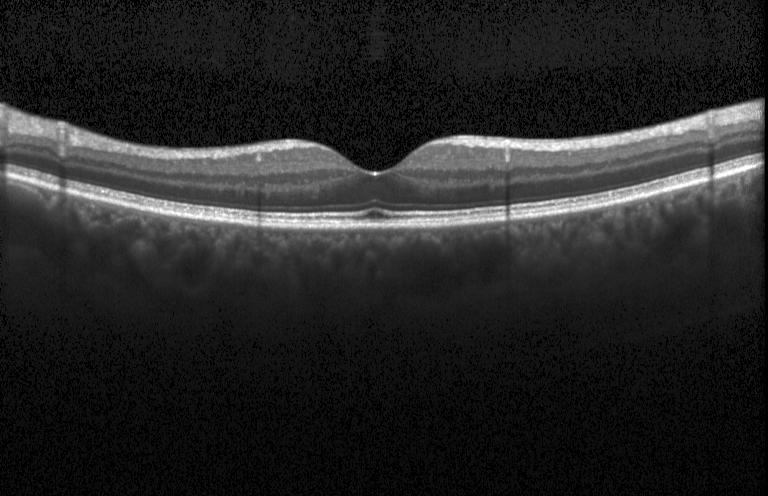
Spectral-domain optical coherence tomography. Centered on the fovea. Instrument: Heidelberg Spectralis. OCT B-scan
No CNV, DME, or drusen.